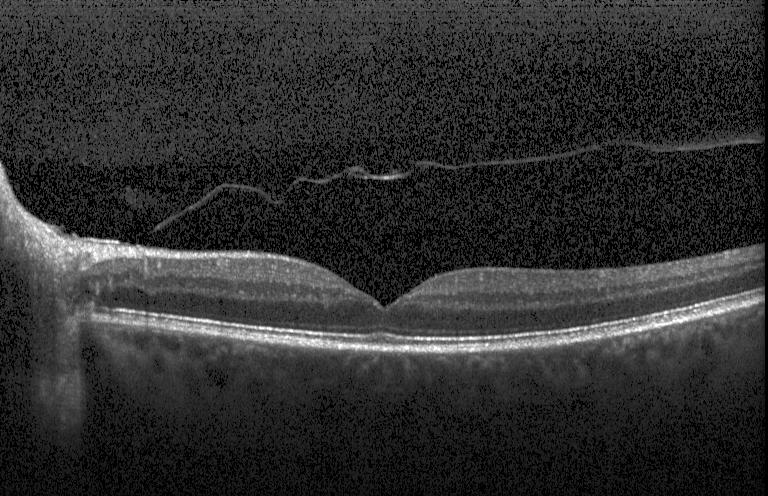
Optical coherence tomography scan; SD-OCT.
Impression: no evidence of choroidal neovascularization, diabetic macular edema, or drusen.